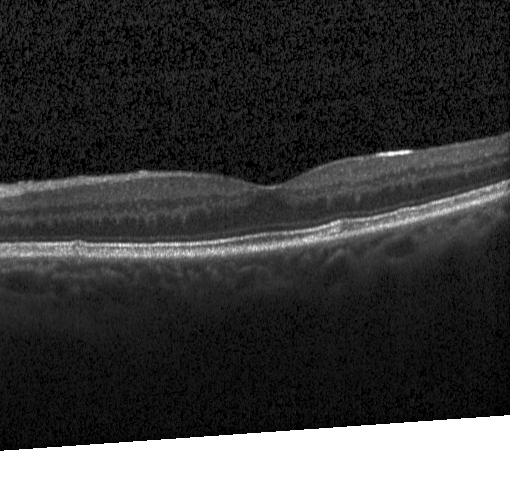
Retinal OCT B-scan; centered on the fovea. Finding: neither choroidal neovascularization, diabetic macular edema, nor drusen.